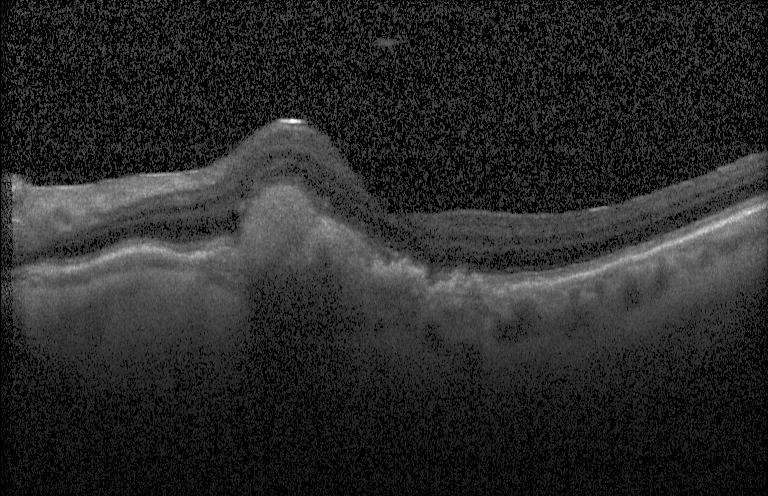 Diagnosis: a choroidal neovascular membrane.